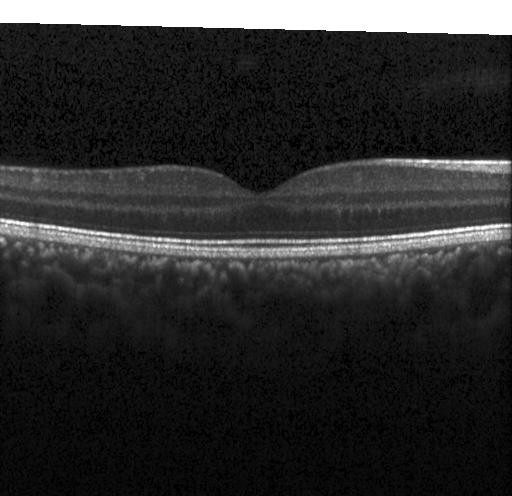
Optical coherence tomography B-scan
This B-scan demonstrates no CNV, DME, or drusen.